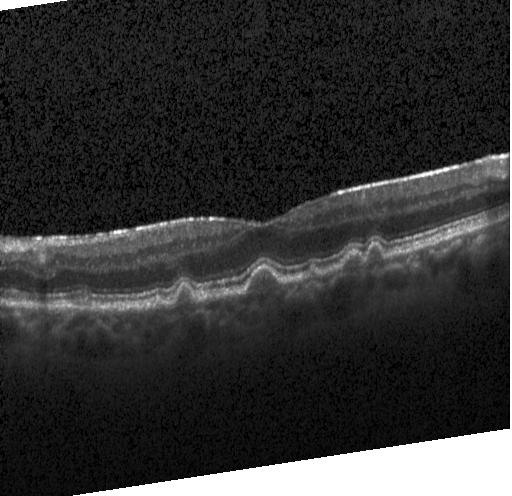
Retinal OCT cross-section showing sub-RPE drusenoid deposits.